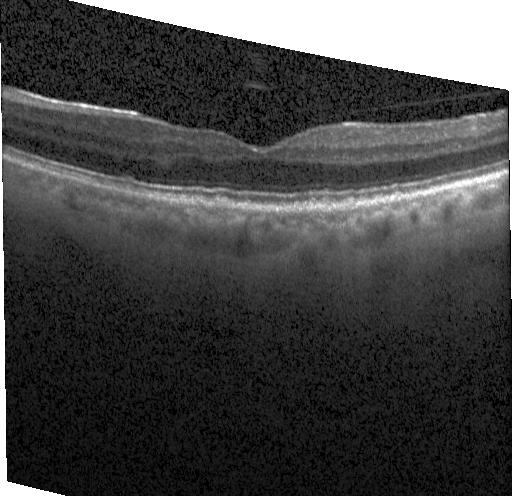
Macular OCT demonstrating drusen.